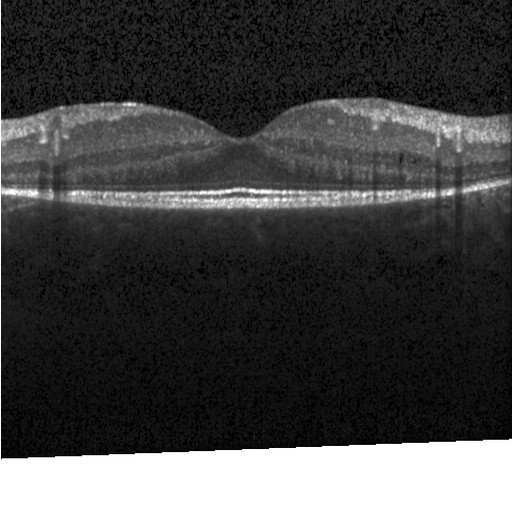
Macular OCT demonstrating DME.